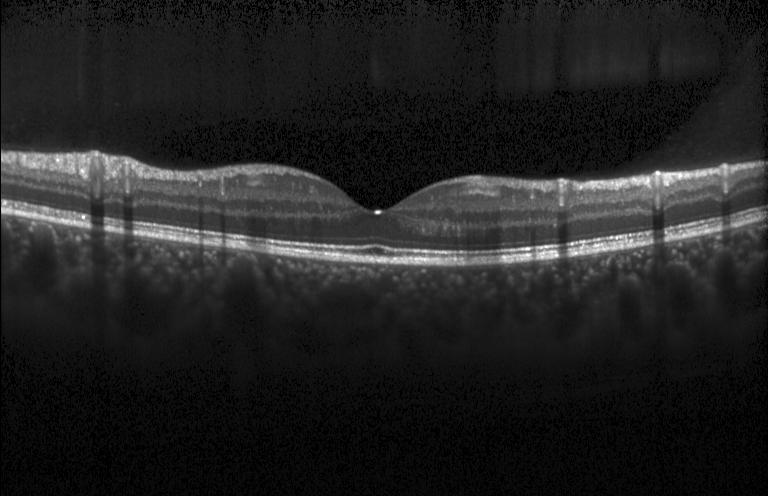

Retinal OCT cross-section showing no CNV, no DME, and no drusen.